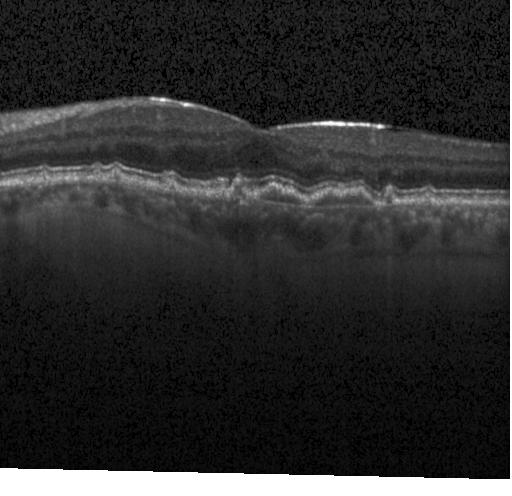
OCT scan showing drusen.